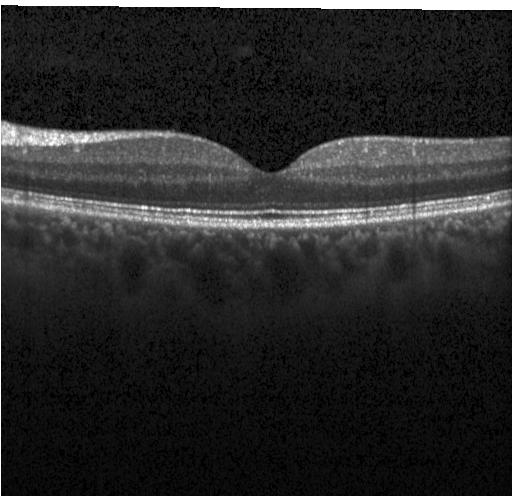
SD-OCT, retinal OCT B-scan. Finding: no evidence of choroidal neovascularization, diabetic macular edema, or drusen.